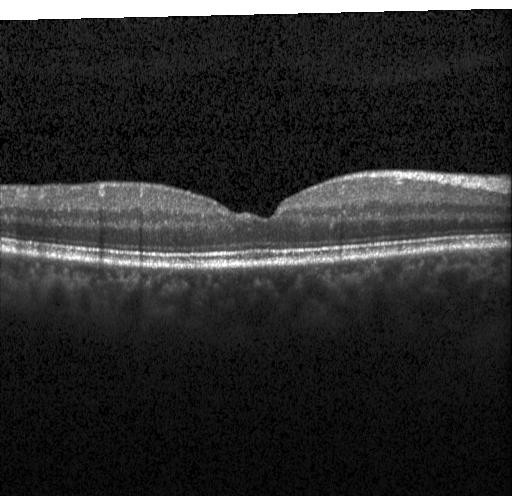
Through the macula, OCT B-scan — Impression: no evidence of choroidal neovascularization, diabetic macular edema, or drusen.